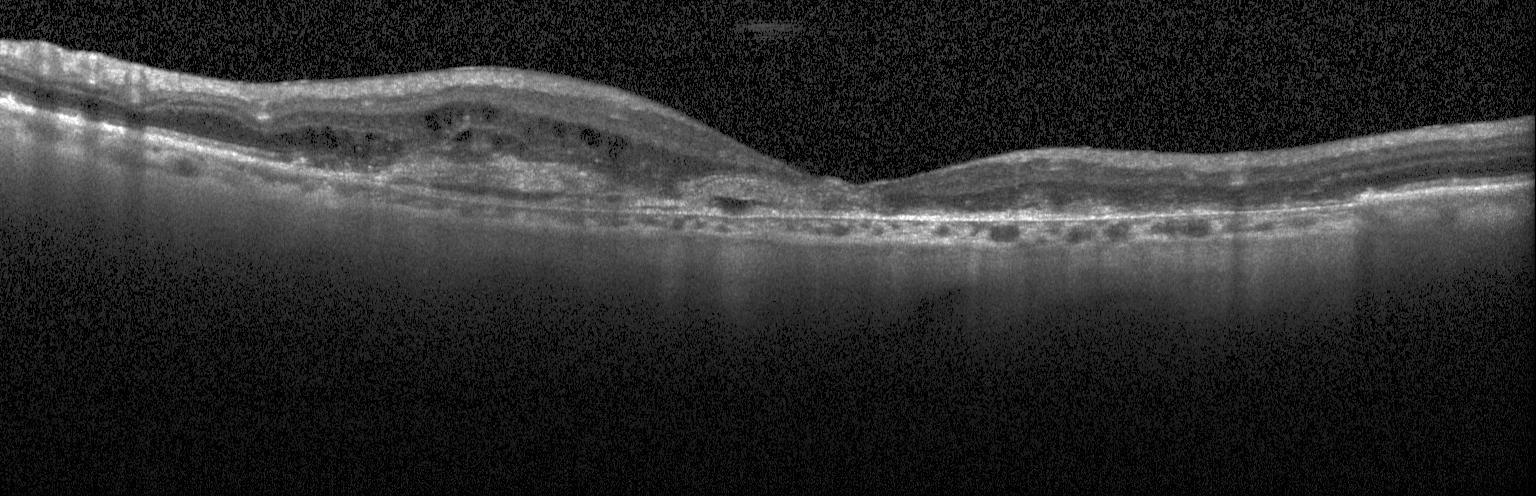
Optical coherence tomography B-scan
Diagnosis: choroidal neovascularization.